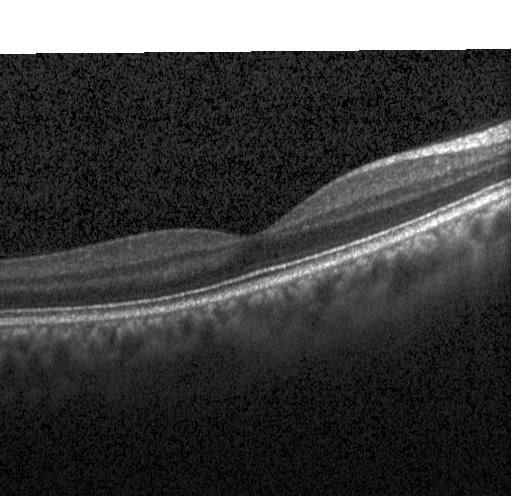 OCT B-scan showing no choroidal neovascularization, diabetic macular edema, or drusen.